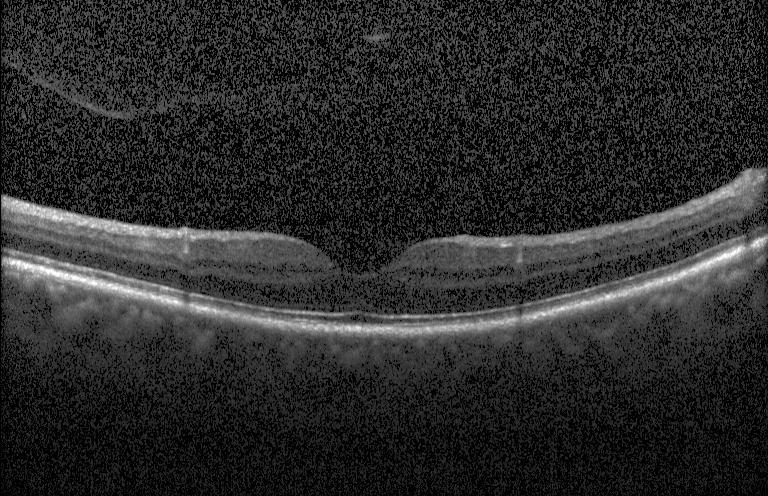 Acquired on a Heidelberg Spectralis; OCT B-scan. Assessment: no evidence of choroidal neovascularization, diabetic macular edema, or drusen.